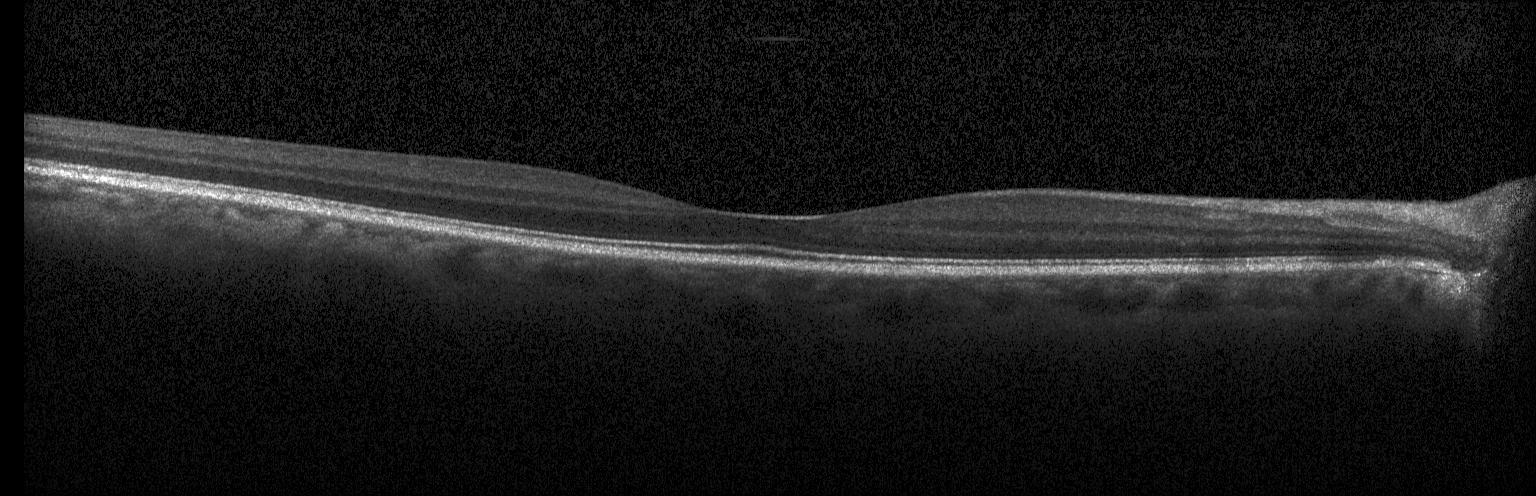 OCT line scan
Diagnosis: no CNV, no DME, and no drusen.